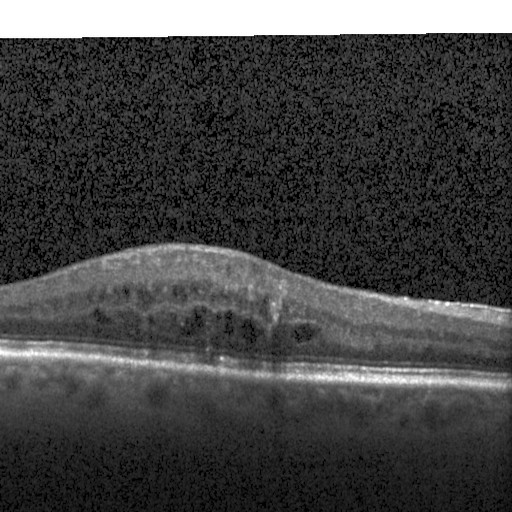
Optical coherence tomography scan.
Finding: diabetic macular edema.